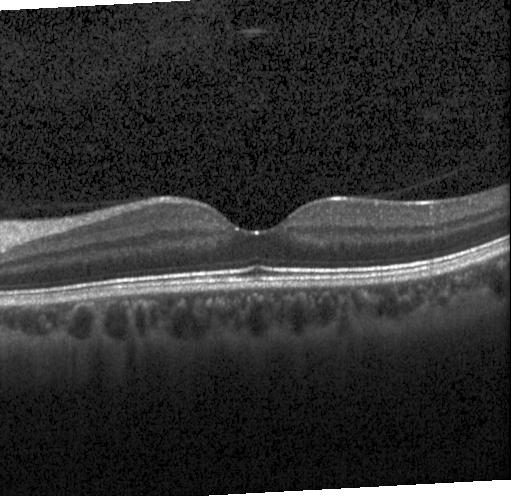

Through the macula, optical coherence tomography scan, acquired on a Heidelberg Spectralis, SD-OCT
Dx: no choroidal neovascularization, no diabetic macular edema, and no drusen.